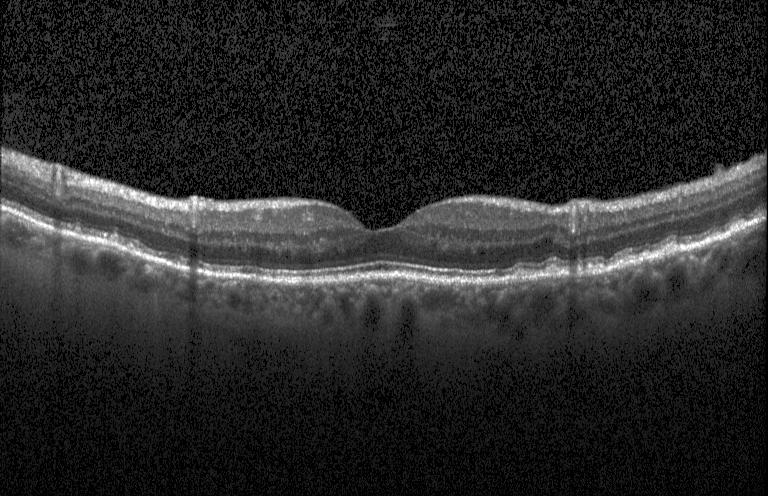

Instrument: Heidelberg Spectralis; spectral-domain optical coherence tomography; macular scan; optical coherence tomography scan. Diagnosis: drusen.